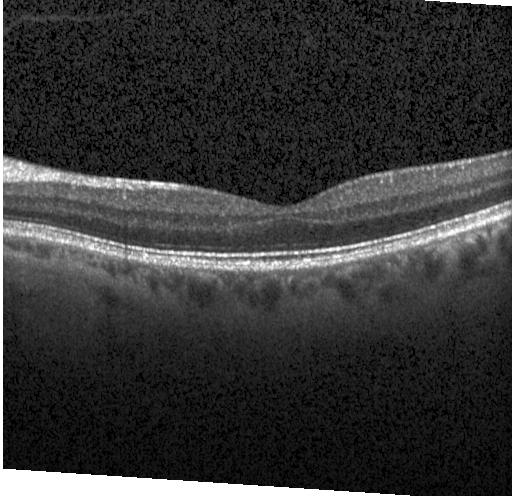

Finding: no evidence of choroidal neovascularization, diabetic macular edema, or drusen.